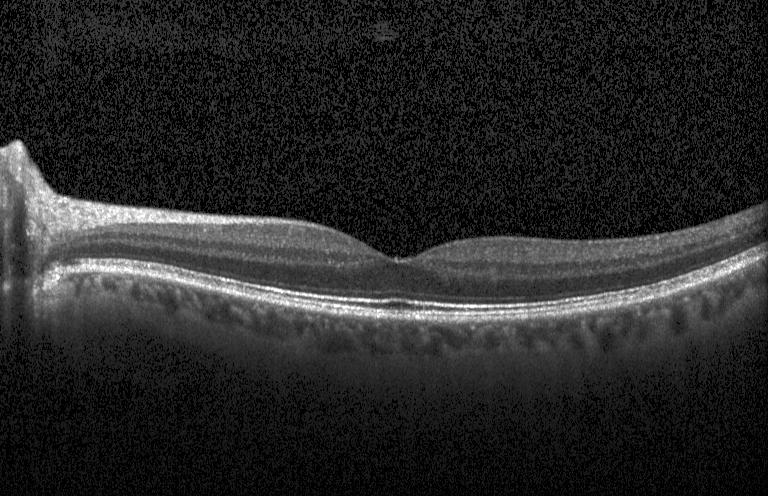
Acquired on a Heidelberg Spectralis · spectral-domain optical coherence tomography · centered on the fovea · optical coherence tomography scan — Impression: neither choroidal neovascularization, diabetic macular edema, nor drusen.